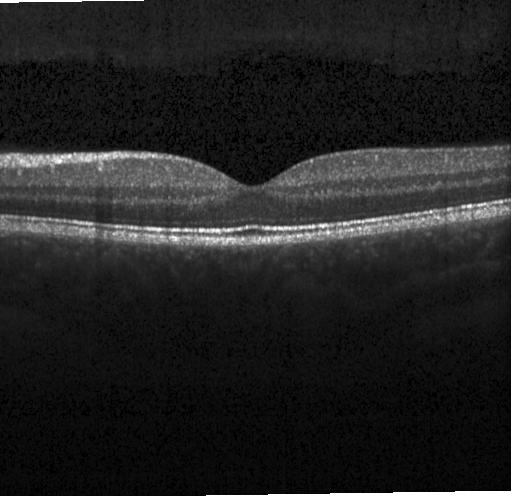

Diagnosis: no evidence of choroidal neovascularization, diabetic macular edema, or drusen.